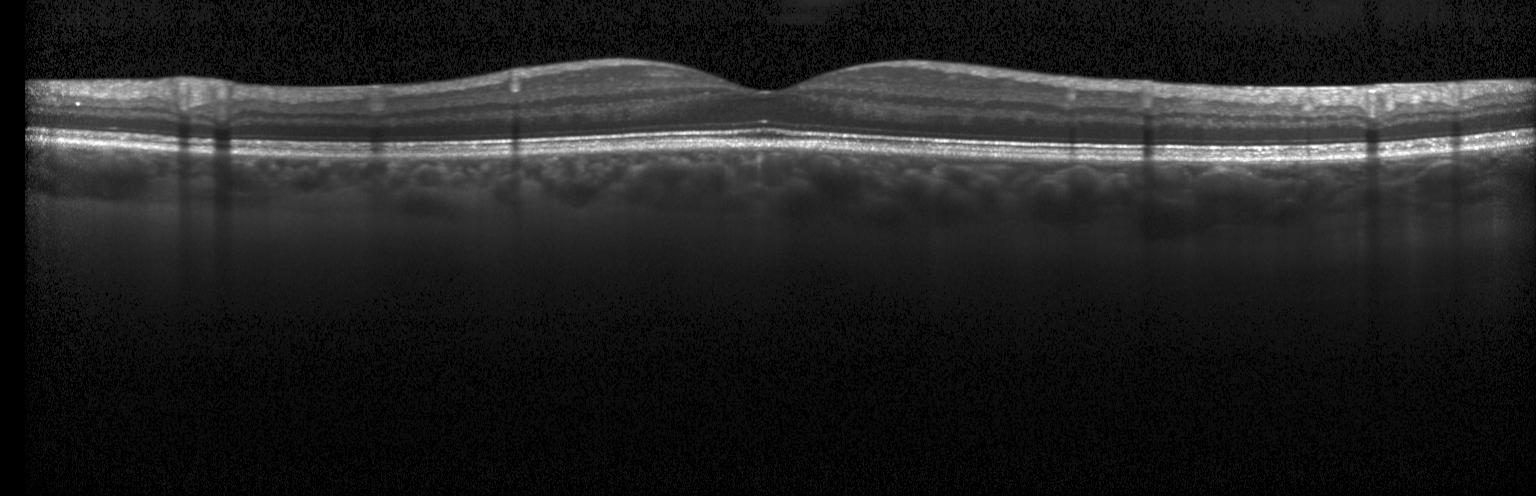
Finding: neither CNV, DME, nor drusen.